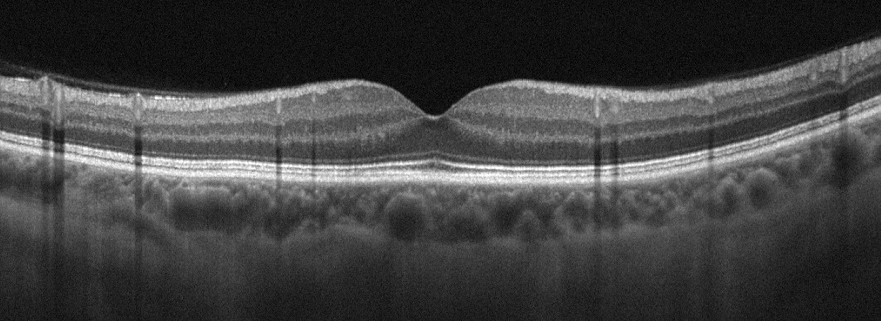 Impression: no AMD, DME, ERM, RAO, RVO, or VID.